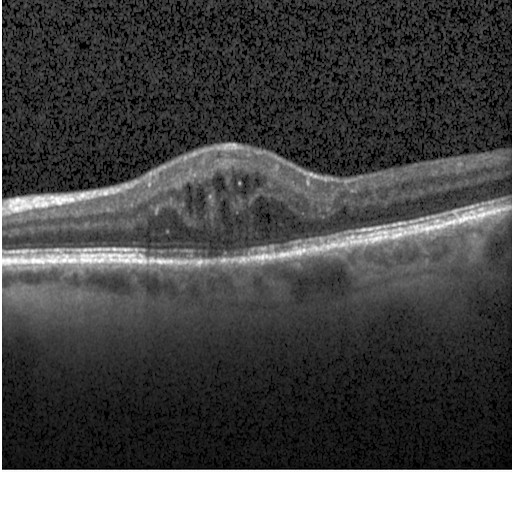
OCT finding: diabetic macular edema (DME).